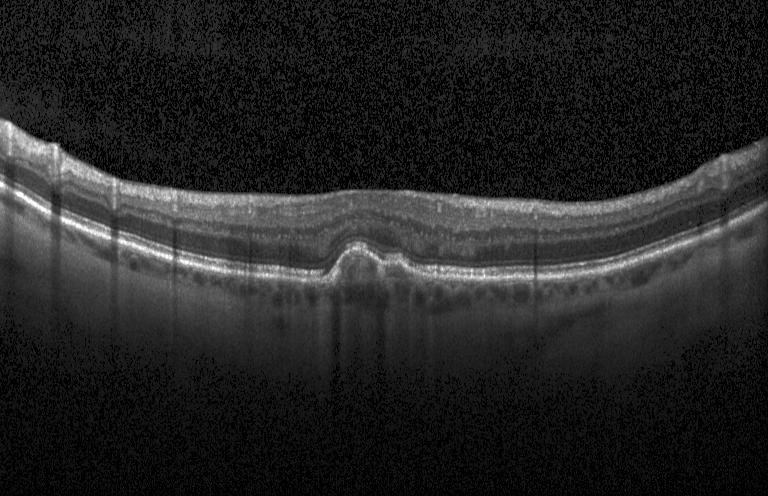
Impression: a choroidal neovascular membrane.